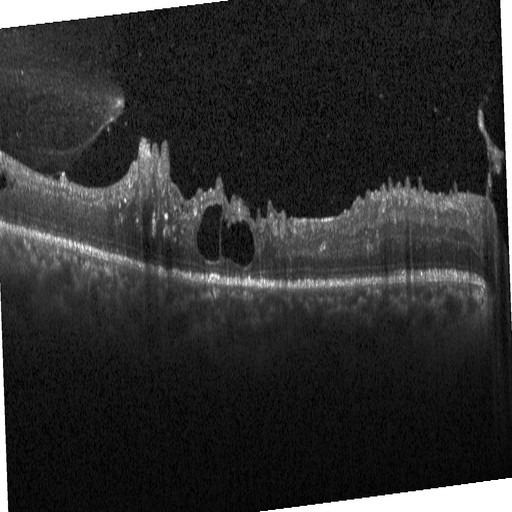

Acquired on a Heidelberg Spectralis; OCT line scan; centered on the fovea; spectral-domain OCT. This B-scan demonstrates DME.